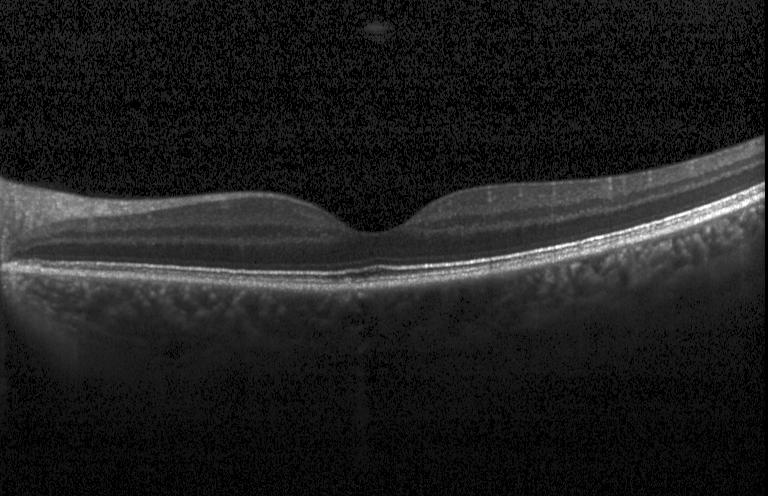
Macular OCT demonstrating no choroidal neovascularization, diabetic macular edema, or drusen.